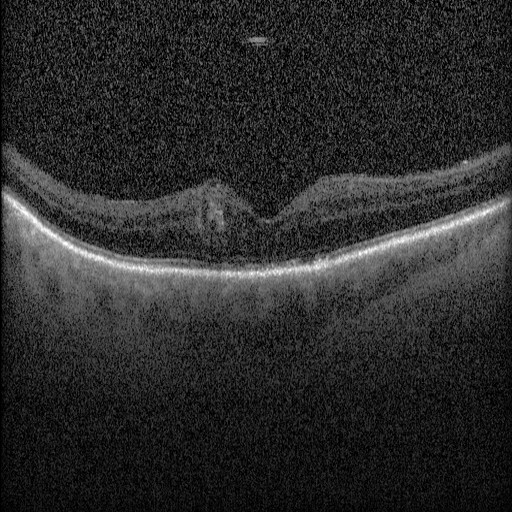 Retinal OCT cross-section. Impression: DME.